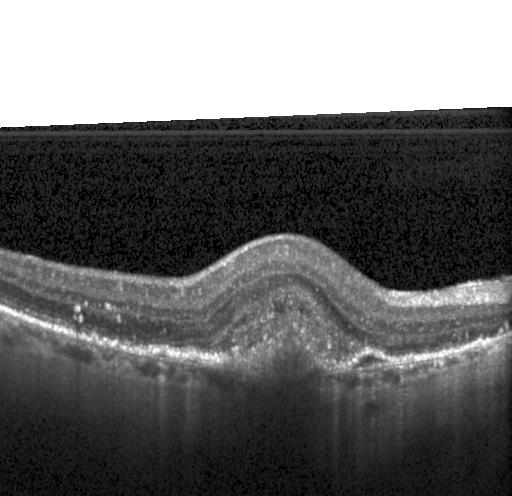
Optical coherence tomography scan. Acquired on a Heidelberg Spectralis. OCT finding: choroidal neovascularization.